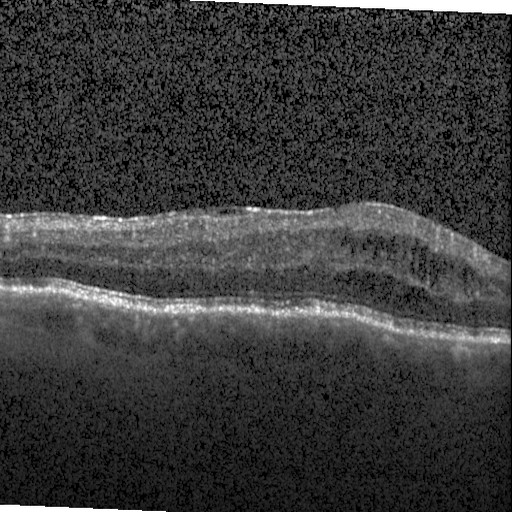

Assessment: diabetic macular edema (DME).